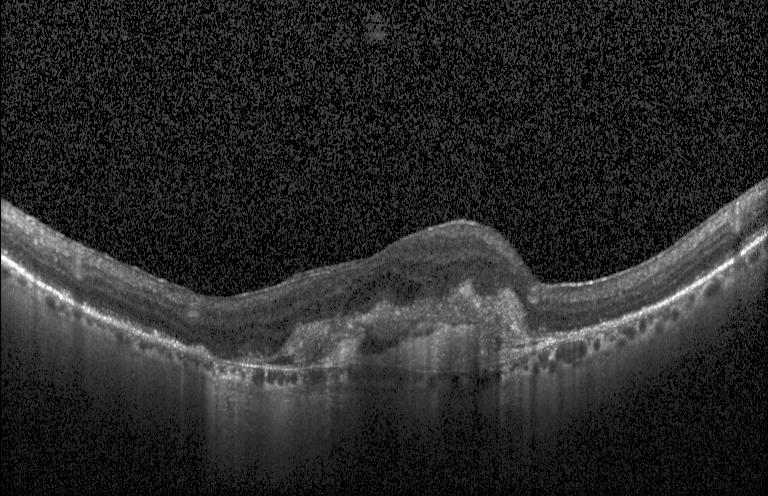

Fovea-centered, Heidelberg Spectralis, spectral-domain OCT, OCT line scan
Finding: a choroidal neovascular membrane.